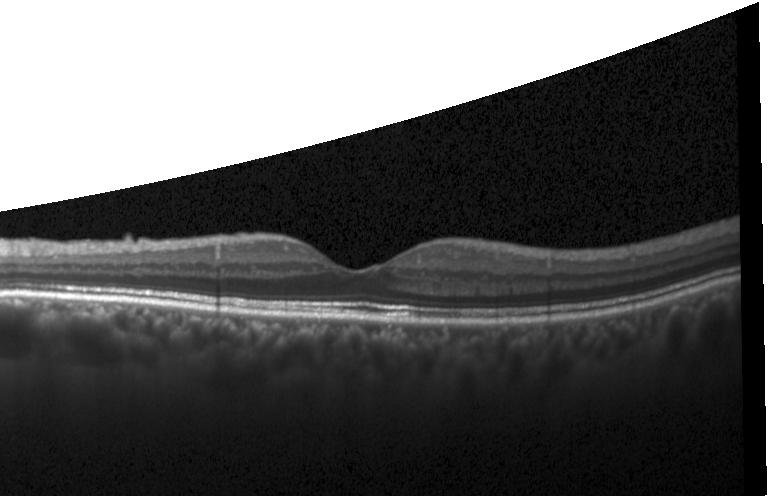

Dx: no evidence of CNV, DME, or drusen.